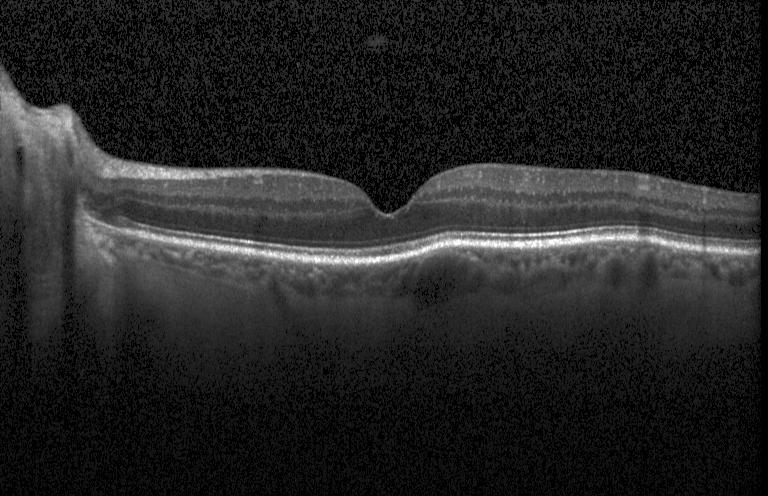

Spectral-domain optical coherence tomography, retinal OCT B-scan, through the macula.
Assessment: no evidence of choroidal neovascularization, diabetic macular edema, or drusen.